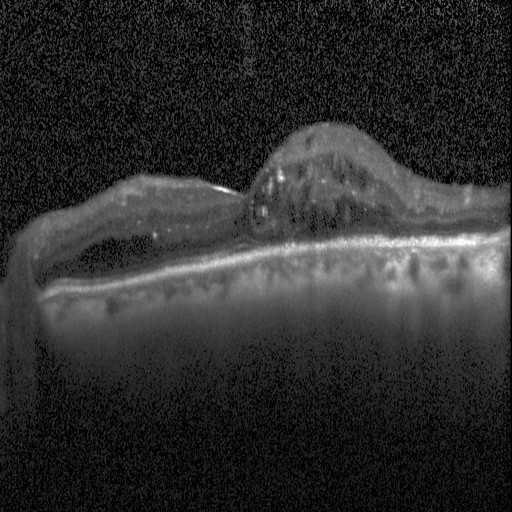

Instrument: Heidelberg Spectralis. Optical coherence tomography B-scan. The scan shows diabetic macular edema.